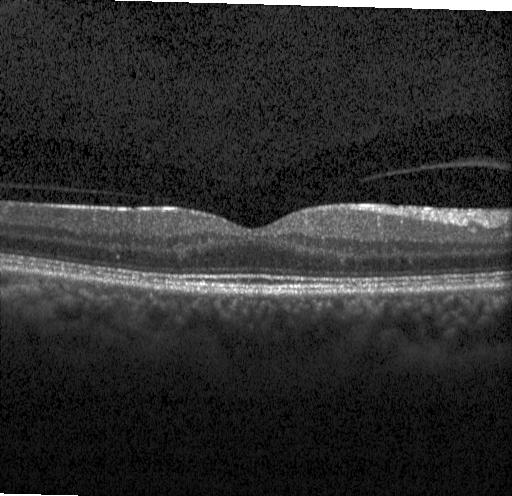

OCT finding: no evidence of CNV, DME, or drusen.